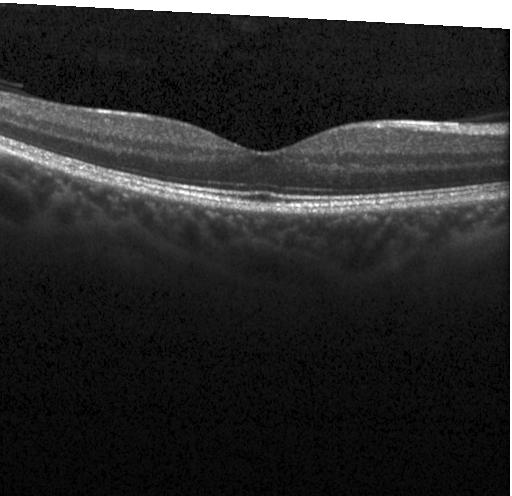 Macular OCT: no CNV, DME, or drusen.